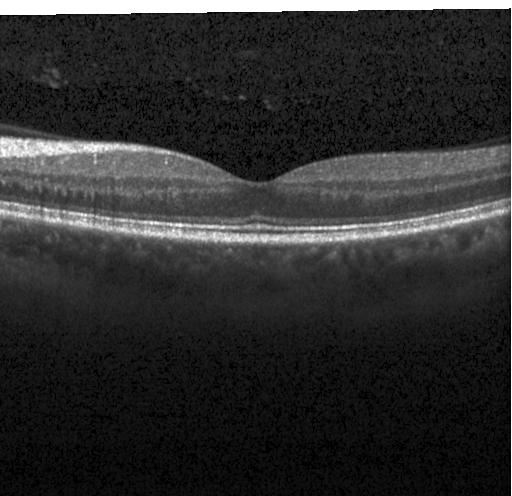
Assessment: no choroidal neovascularization, no diabetic macular edema, and no drusen.